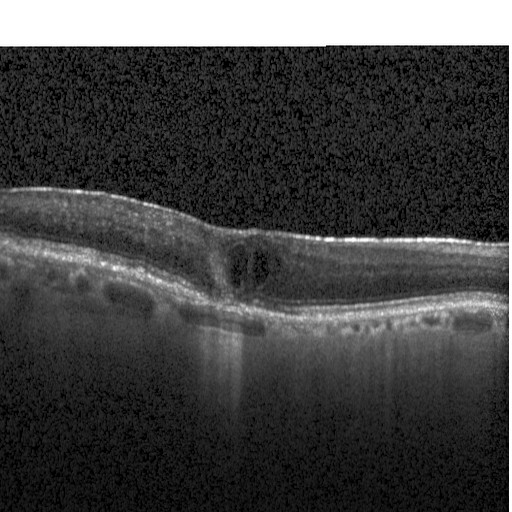

Impression: diabetic macular edema.